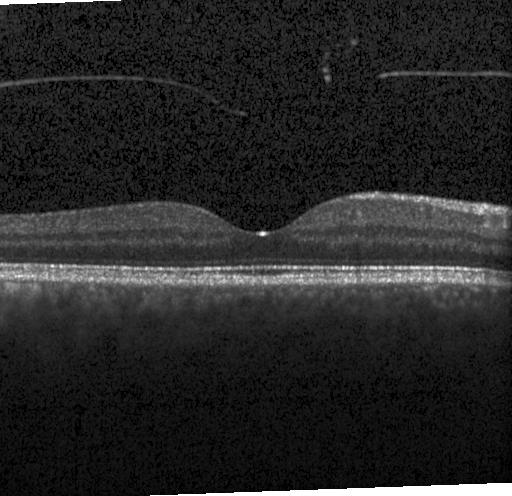 Acquired on a Heidelberg Spectralis · spectral-domain optical coherence tomography · retinal OCT B-scan.
OCT finding: no choroidal neovascularization, no diabetic macular edema, and no drusen.